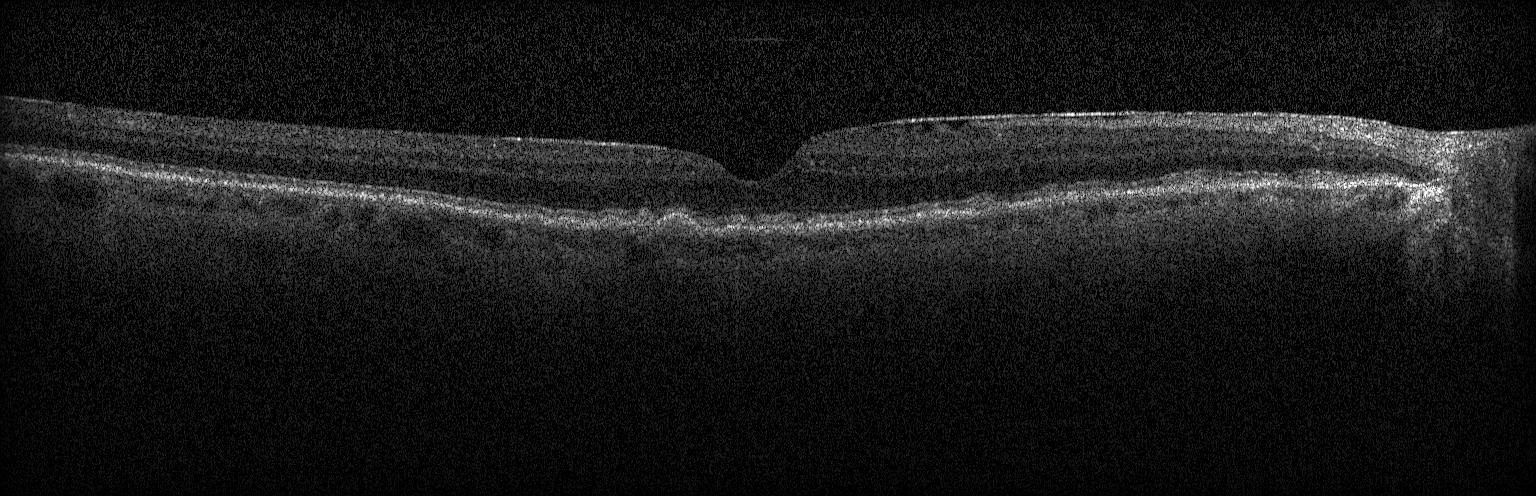 SD-OCT. Optical coherence tomography scan. Macular scan. Heidelberg Spectralis.
Impression: multiple drusen.